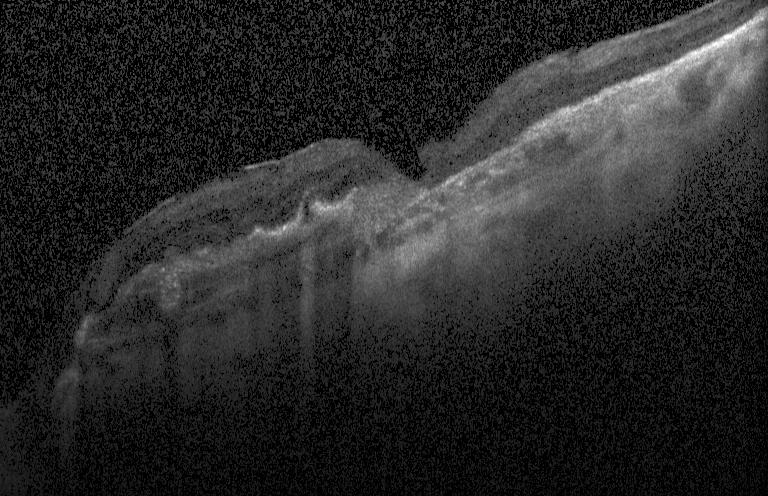 OCT line scan · macular scan.
The scan shows choroidal neovascularization (CNV).